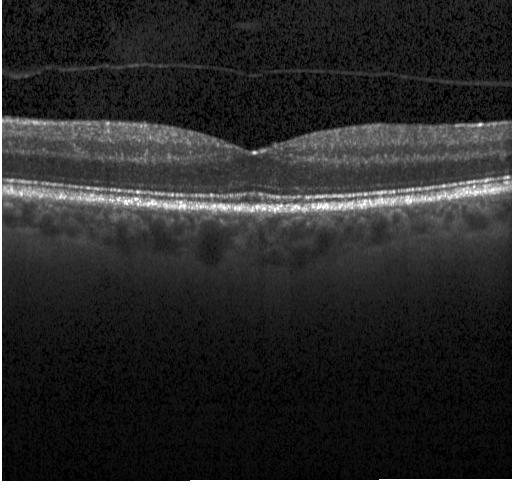

Optical coherence tomography B-scan
This B-scan demonstrates neither CNV, DME, nor drusen.